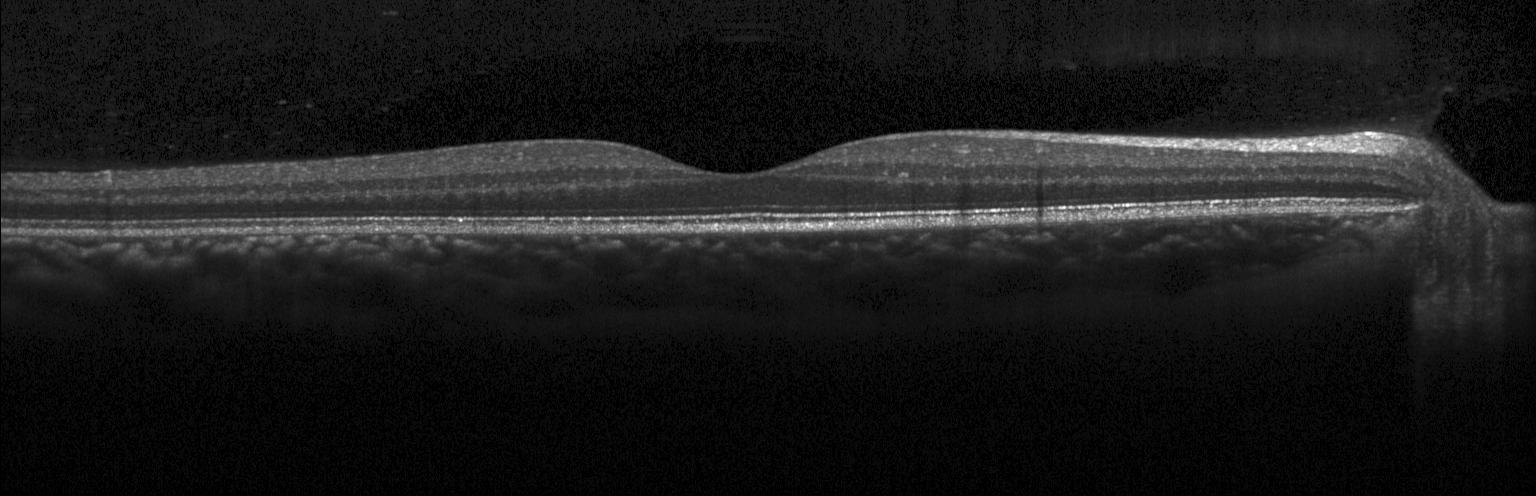

OCT line scan. Fovea-centered
Dx: no evidence of CNV, DME, or drusen.